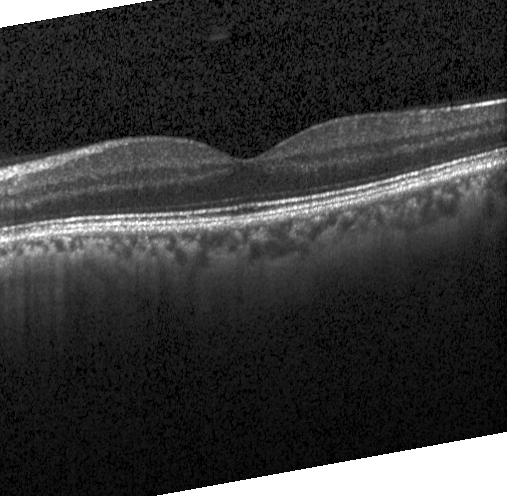 OCT B-scan showing no choroidal neovascularization, diabetic macular edema, or drusen.